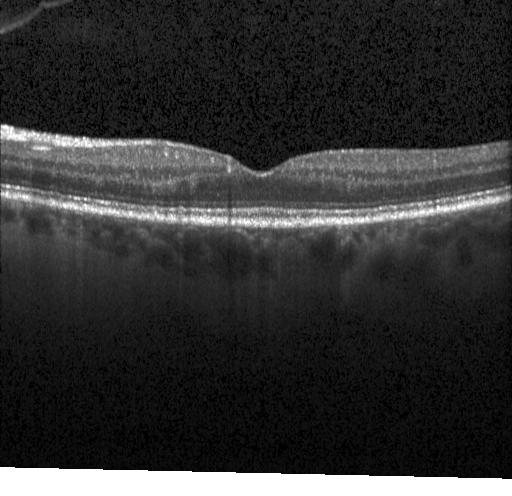
OCT line scan · acquired on a Heidelberg Spectralis.
Impression: no CNV, DME, or drusen.